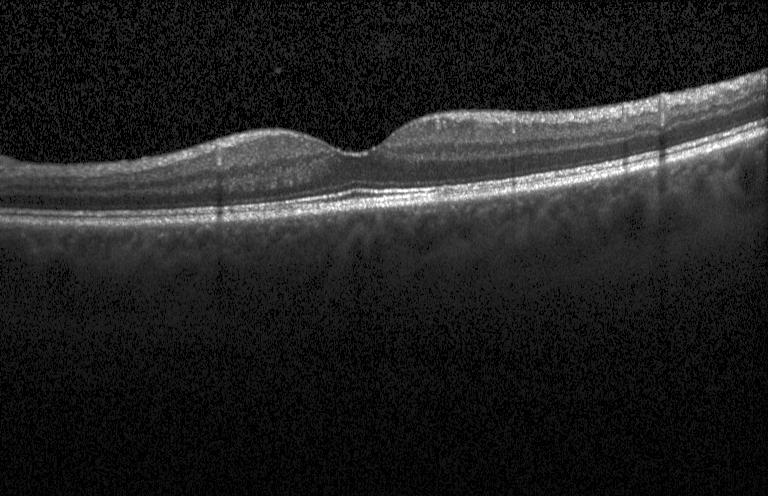

OCT scan showing no choroidal neovascularization, diabetic macular edema, or drusen.